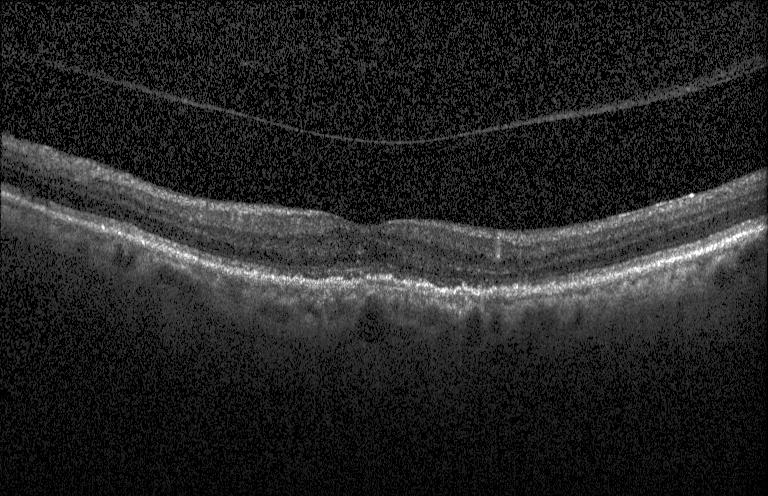
OCT B-scan; through the macula; instrument: Heidelberg Spectralis — This B-scan demonstrates a choroidal neovascular membrane.